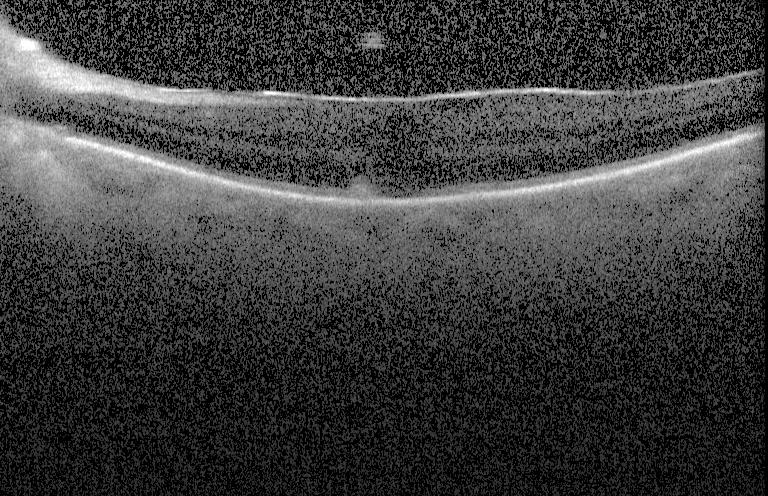 Dx: multiple drusen.